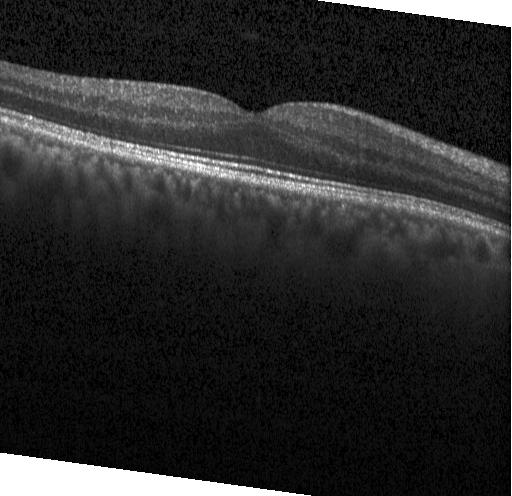
OCT B-scan showing no CNV, no DME, and no drusen.